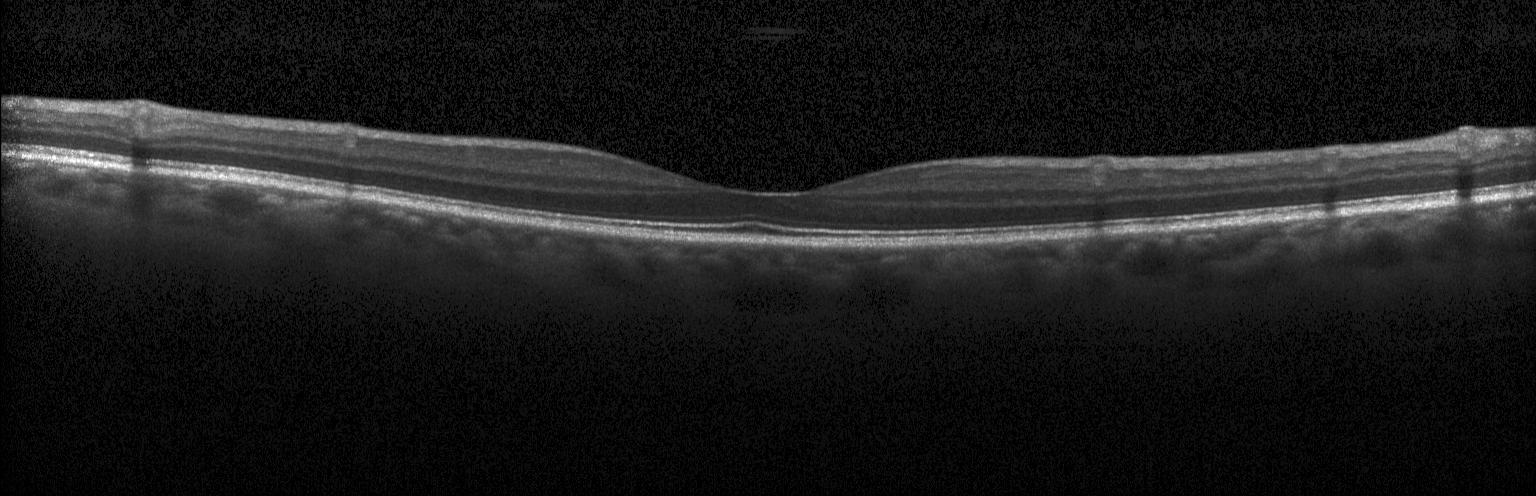 Retinal OCT B-scan · horizontal scan through the fovea
Macular OCT: neither CNV, DME, nor drusen.